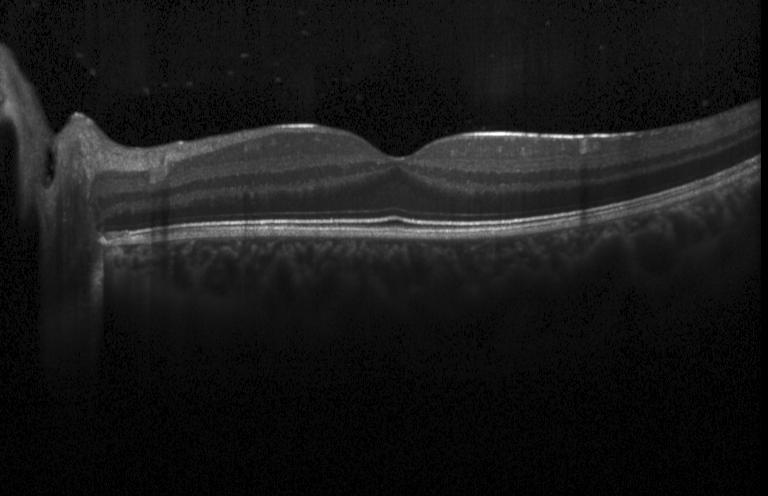
Spectral-domain OCT. OCT B-scan. Centered on the fovea.
Macular OCT: no evidence of choroidal neovascularization, diabetic macular edema, or drusen.